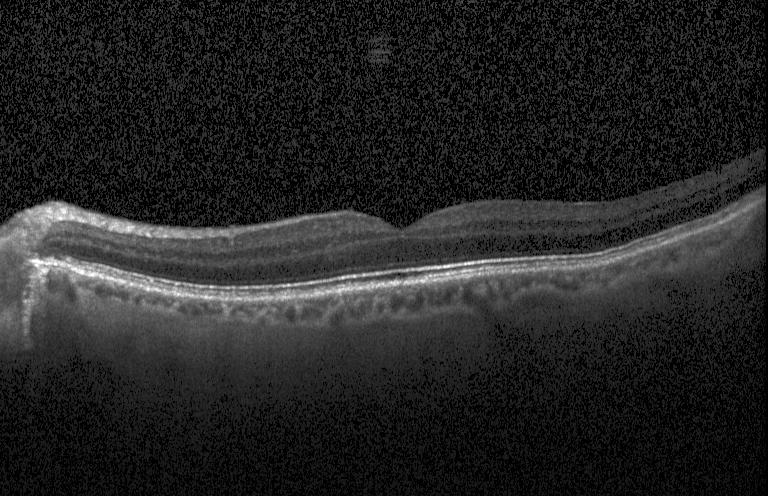
OCT finding: no choroidal neovascularization, diabetic macular edema, or drusen.